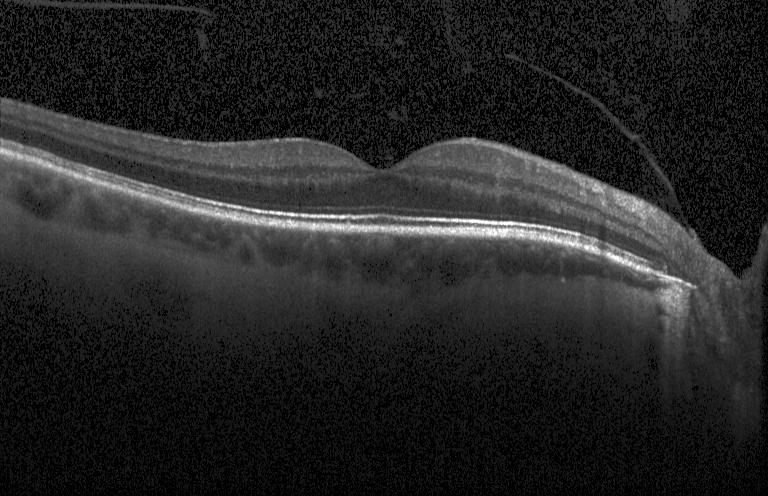
OCT B-scan. Acquired on a Heidelberg Spectralis. Spectral-domain optical coherence tomography. Assessment: no CNV, DME, or drusen.